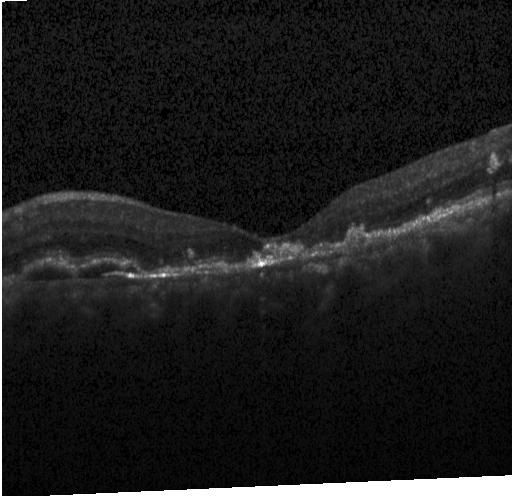

Macular OCT: choroidal neovascularization.